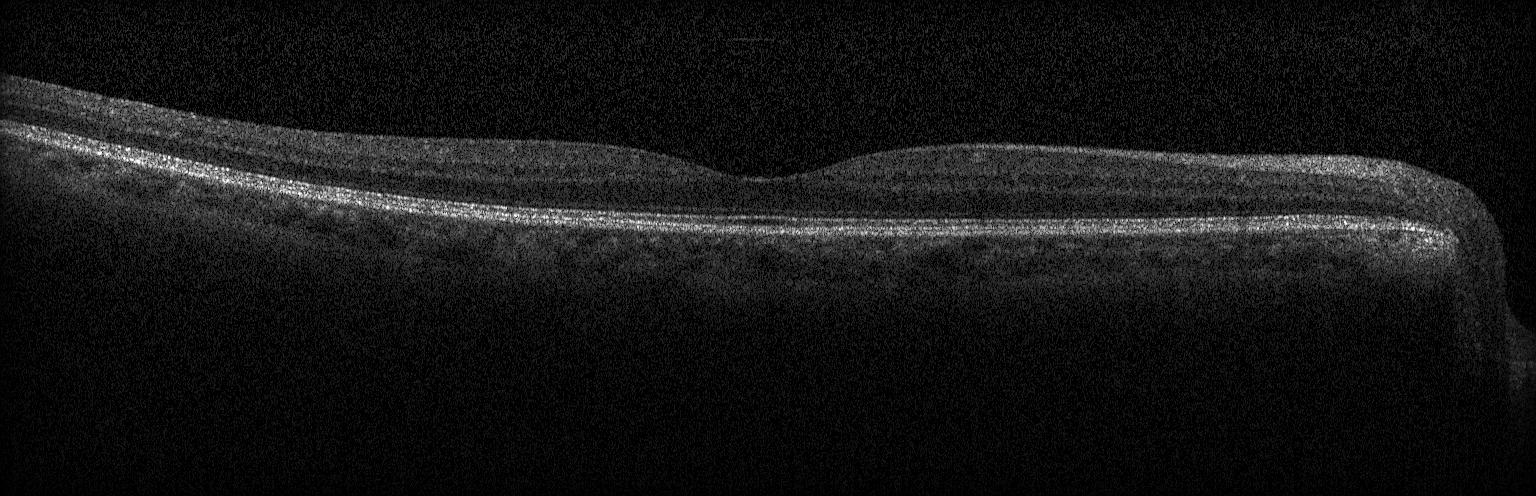 OCT line scan. Impression: no choroidal neovascularization, no diabetic macular edema, and no drusen.